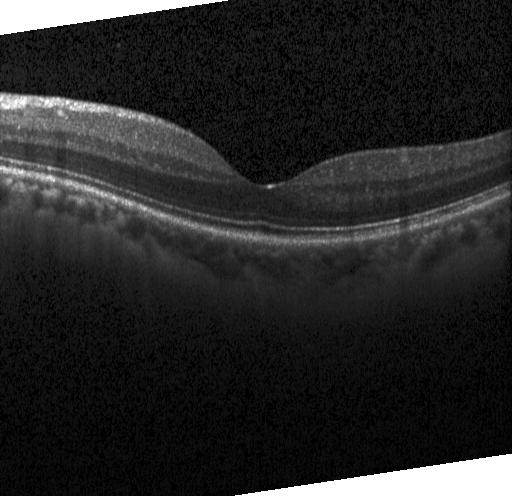
Retinal OCT B-scan
Diagnosis: neither CNV, DME, nor drusen.